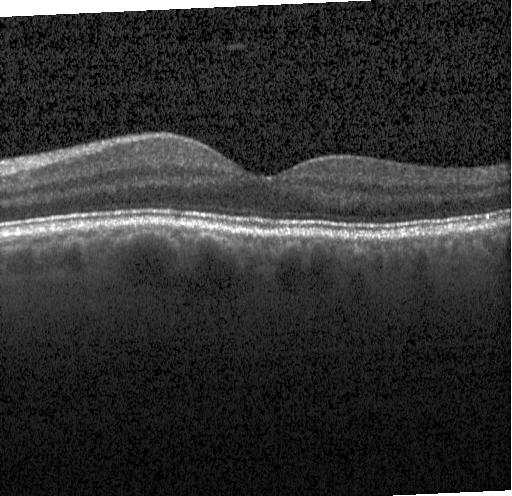

OCT B-scan showing no choroidal neovascularization, no diabetic macular edema, and no drusen.